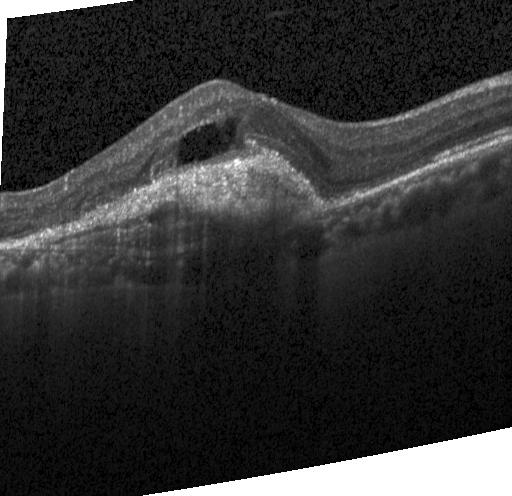

Spectral-domain optical coherence tomography · optical coherence tomography B-scan · Heidelberg Spectralis
Diagnosis: a choroidal neovascular membrane.